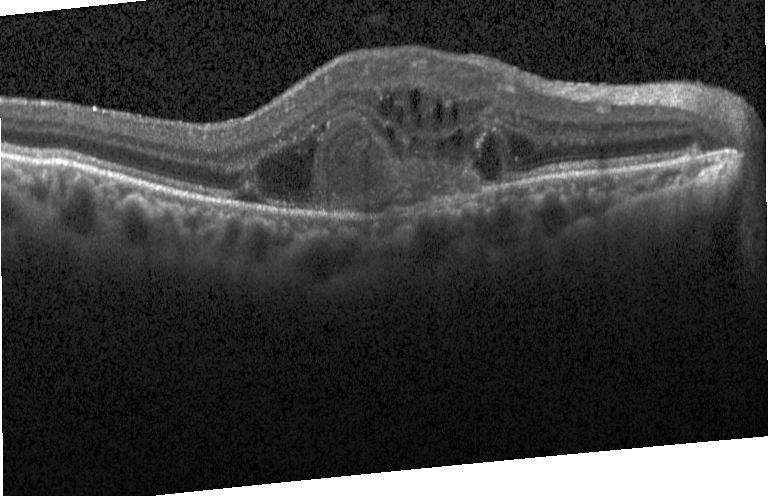
Optical coherence tomography B-scan — Diagnosis: a choroidal neovascular membrane.